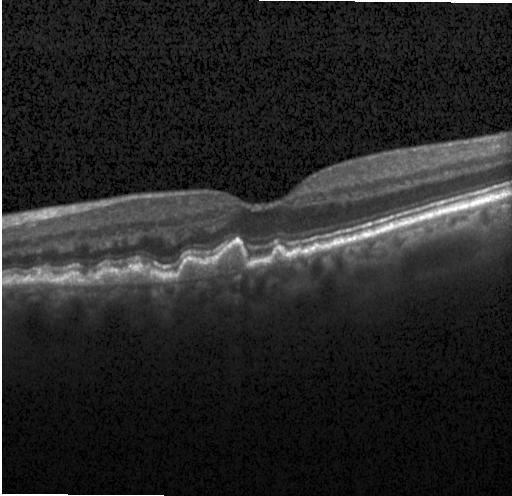
Finding: sub-RPE drusenoid deposits.